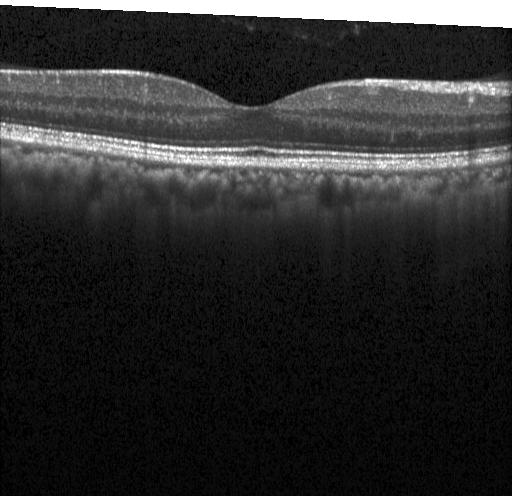

Neither CNV, DME, nor drusen.